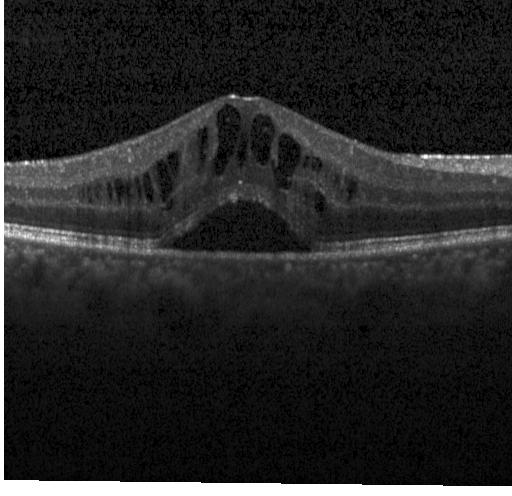

OCT B-scan
Assessment: DME.